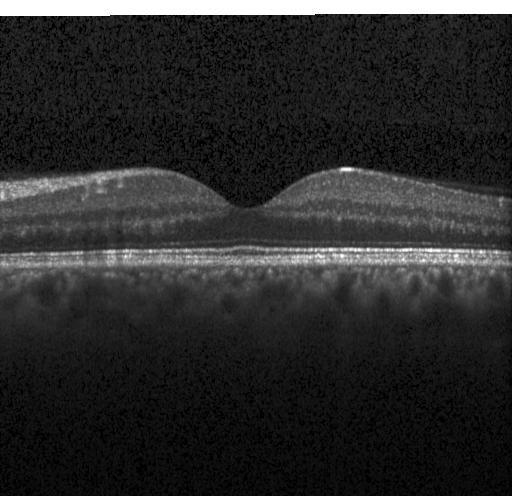

Fovea-centered. Heidelberg Spectralis OCT system. Retinal OCT B-scan
Dx: no evidence of choroidal neovascularization, diabetic macular edema, or drusen.